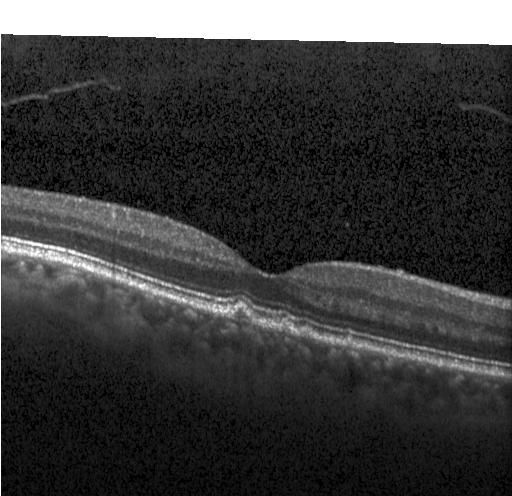
Diagnosis: sub-RPE drusenoid deposits.